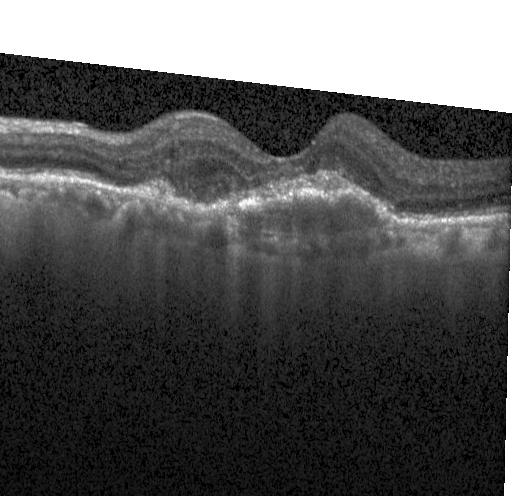

OCT B-scan showing a choroidal neovascular membrane.